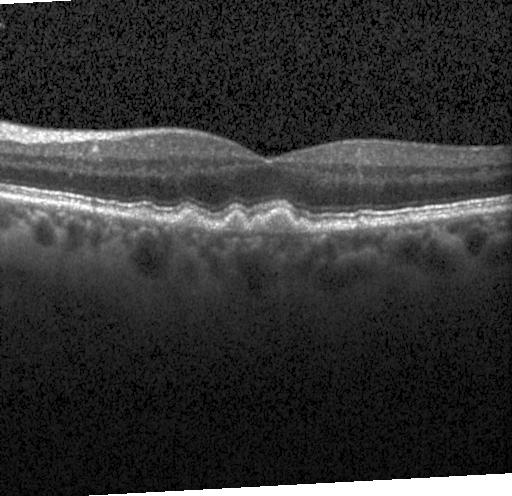
Optical coherence tomography scan.
This B-scan demonstrates sub-RPE drusenoid deposits.